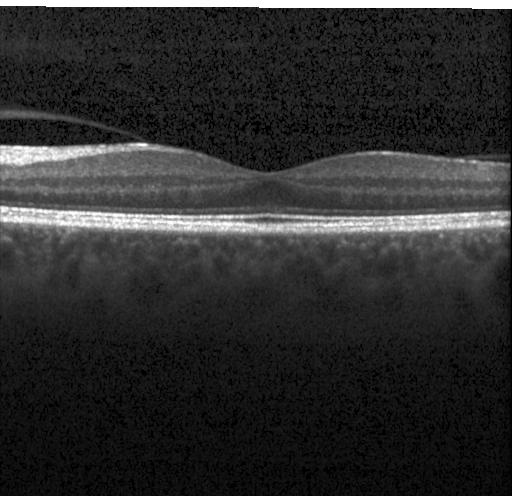

OCT B-scan
This B-scan demonstrates neither CNV, DME, nor drusen.